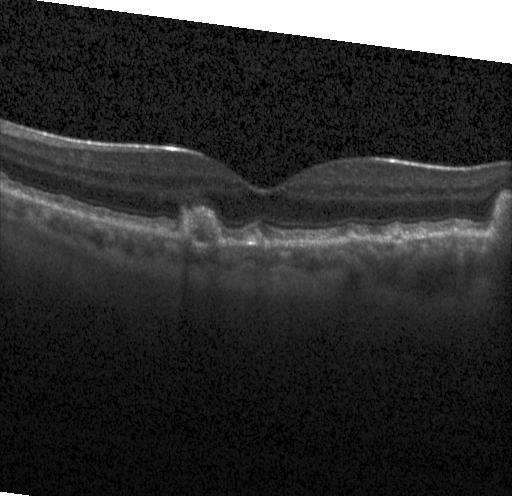
OCT B-scan. Horizontal scan through the fovea. Dx: choroidal neovascularization.